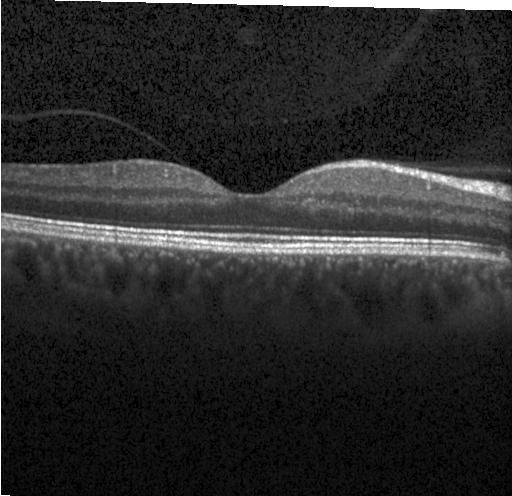
Spectral-domain OCT B-scan: no choroidal neovascularization, no diabetic macular edema, and no drusen.